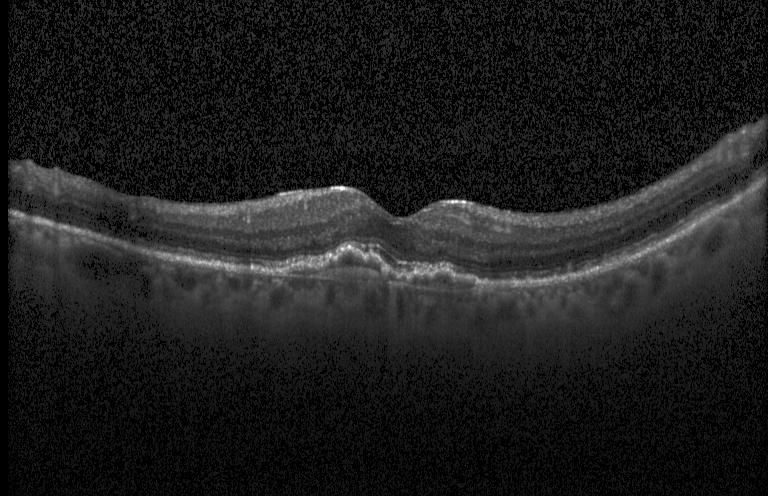

Instrument: Heidelberg Spectralis; spectral-domain optical coherence tomography; OCT line scan. Finding: a choroidal neovascular membrane.